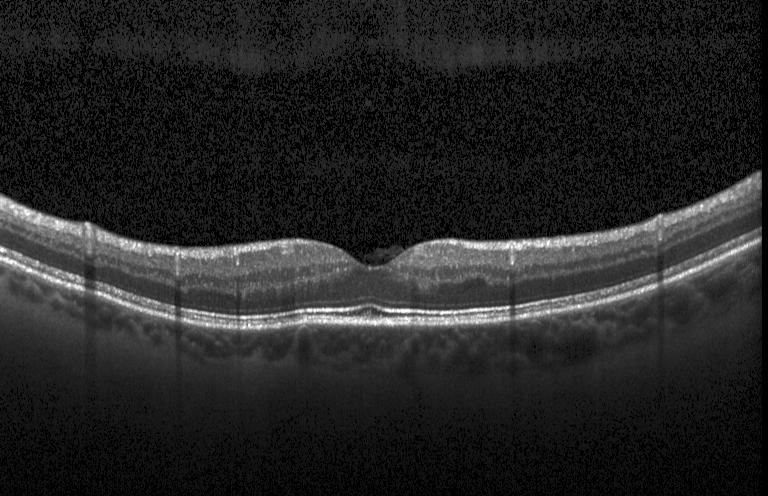 Dx: no choroidal neovascularization, diabetic macular edema, or drusen.